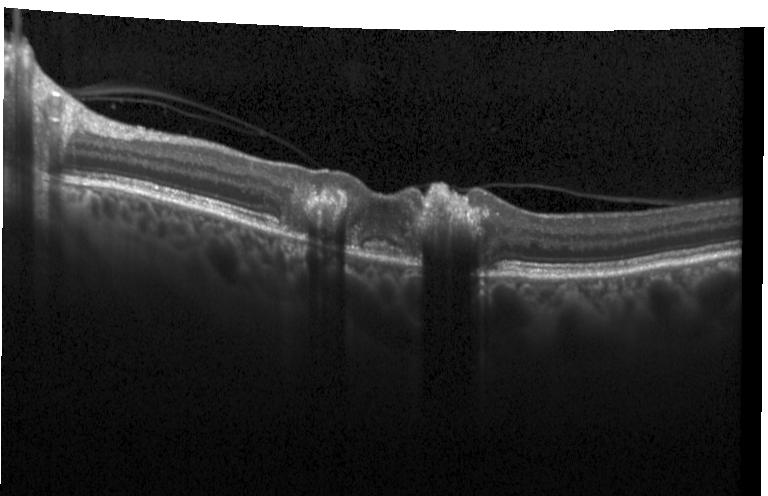
Heidelberg Spectralis OCT system. Fovea-centered. OCT B-scan — This B-scan demonstrates CNV.